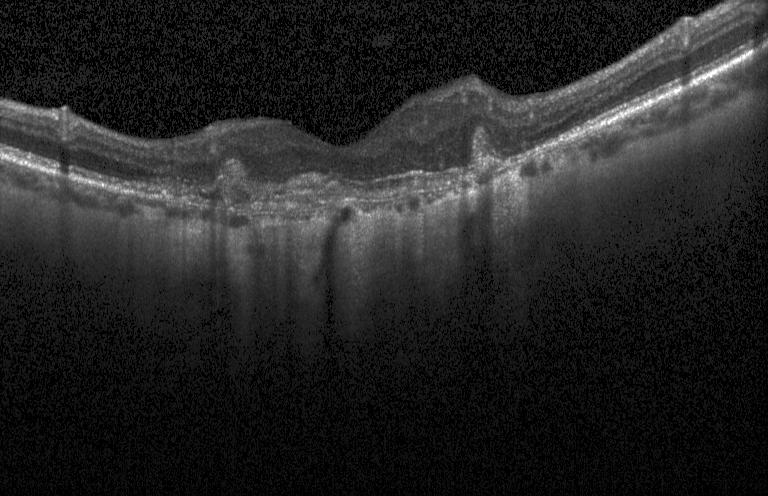

Instrument: Heidelberg Spectralis, spectral-domain OCT, OCT B-scan — OCT finding: a choroidal neovascular membrane.